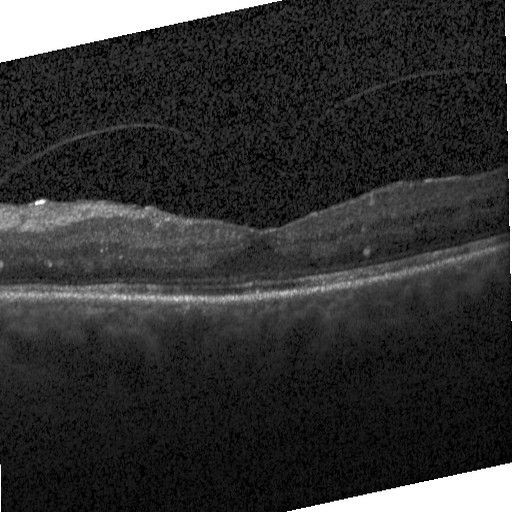 Finding: diabetic macular edema.